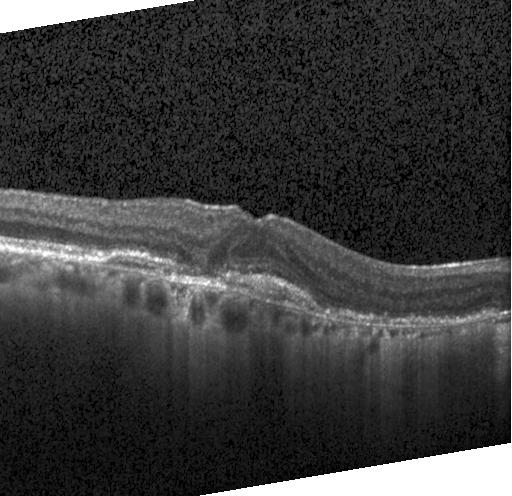

Heidelberg Spectralis · OCT line scan
The scan shows CNV.